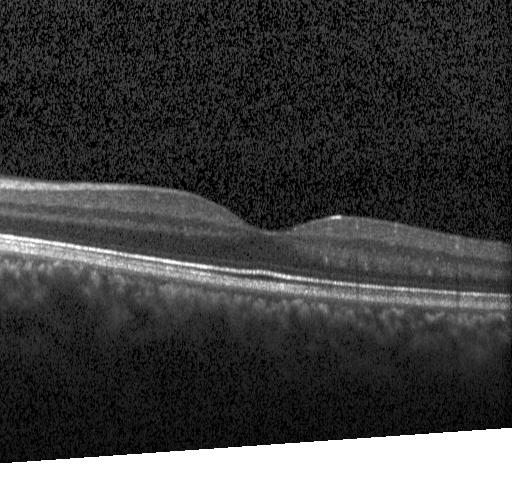
Assessment: no choroidal neovascularization, no diabetic macular edema, and no drusen.